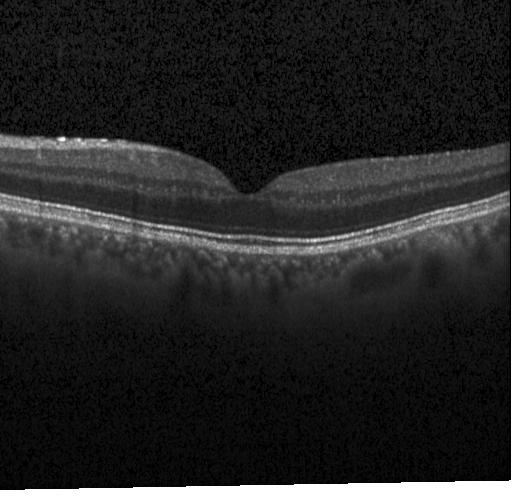
Dx: no evidence of CNV, DME, or drusen.